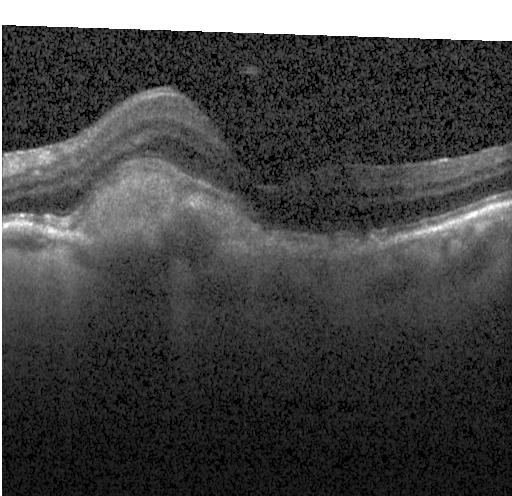 Optical coherence tomography scan. Dx: choroidal neovascularization.